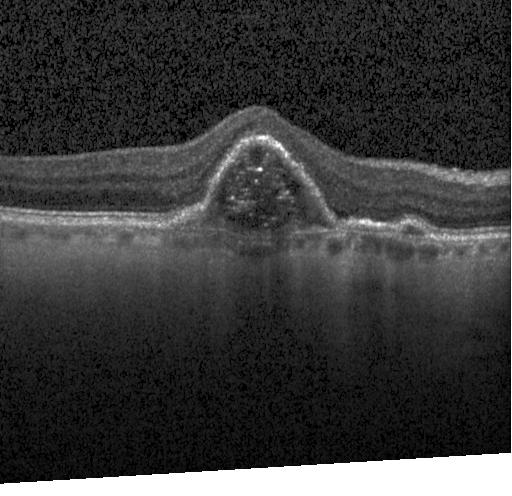 OCT line scan. Fovea-centered. Heidelberg Spectralis. Spectral-domain OCT.
Assessment: choroidal neovascularization (CNV).